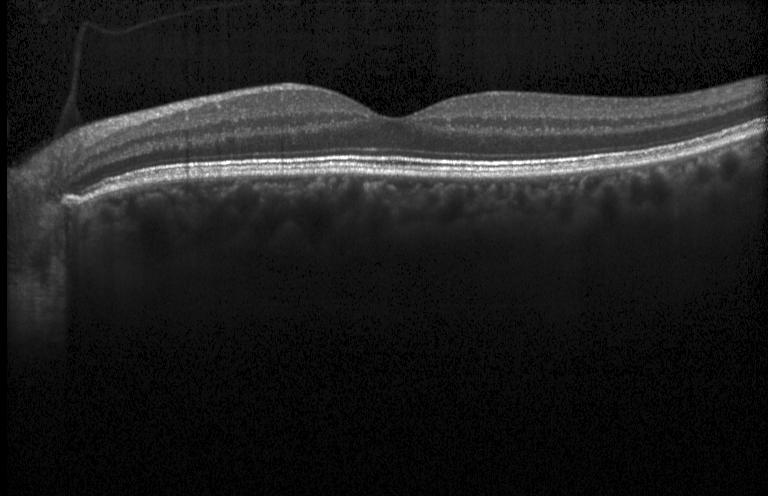 Dx: neither CNV, DME, nor drusen.